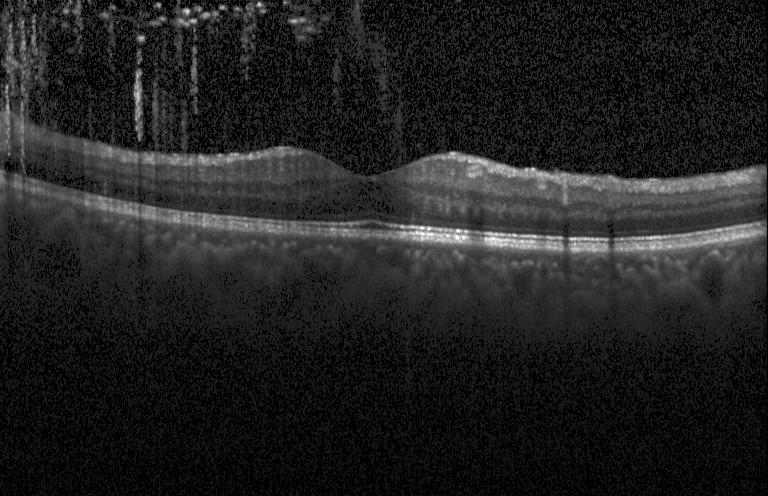

Macular scan. Acquired on a Heidelberg Spectralis. Optical coherence tomography B-scan. SD-OCT — Impression: no evidence of choroidal neovascularization, diabetic macular edema, or drusen.